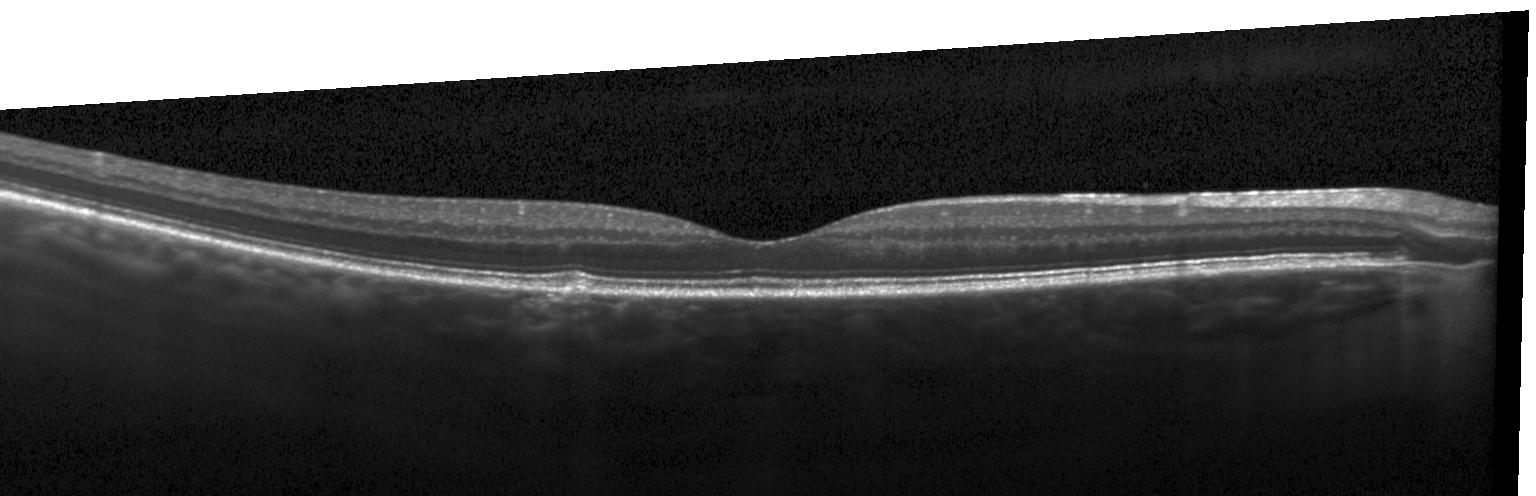
Impression: no choroidal neovascularization, no diabetic macular edema, and no drusen.